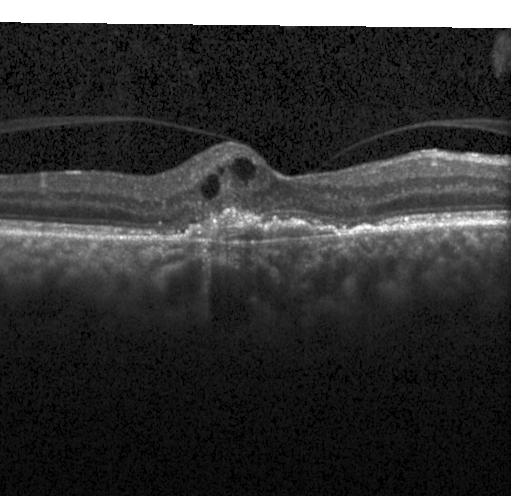

Spectral-domain OCT; optical coherence tomography scan — Assessment: choroidal neovascularization (CNV).